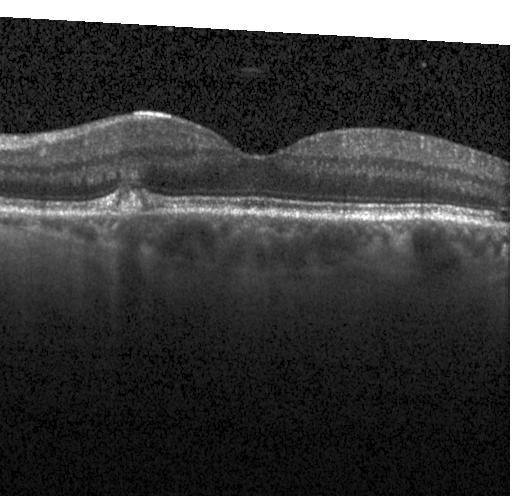
Horizontal scan through the fovea · Heidelberg Spectralis · spectral-domain OCT · OCT line scan. Assessment: sub-RPE drusenoid deposits.